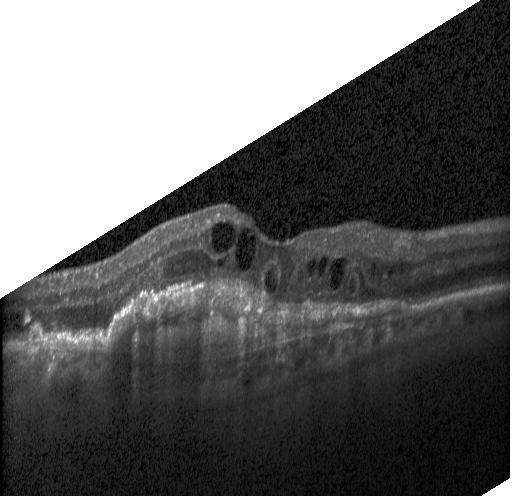
Macular scan; SD-OCT; retinal OCT B-scan.
This B-scan demonstrates choroidal neovascularization (CNV).